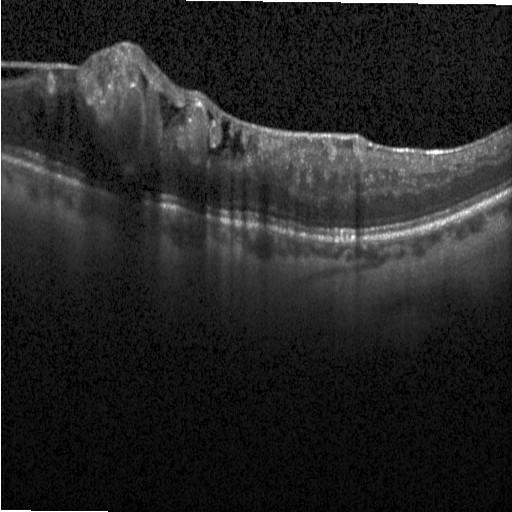

Impression: diabetic macular edema.